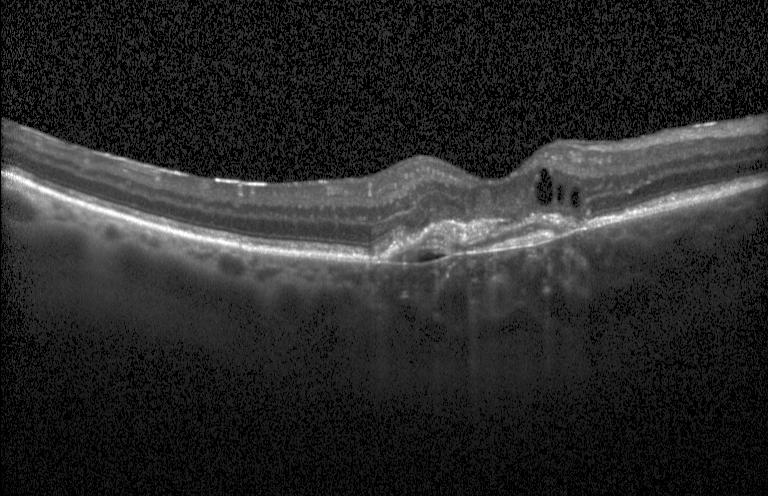 Optical coherence tomography B-scan, Heidelberg Spectralis OCT system, horizontal scan through the fovea, spectral-domain optical coherence tomography. OCT finding: choroidal neovascularization.